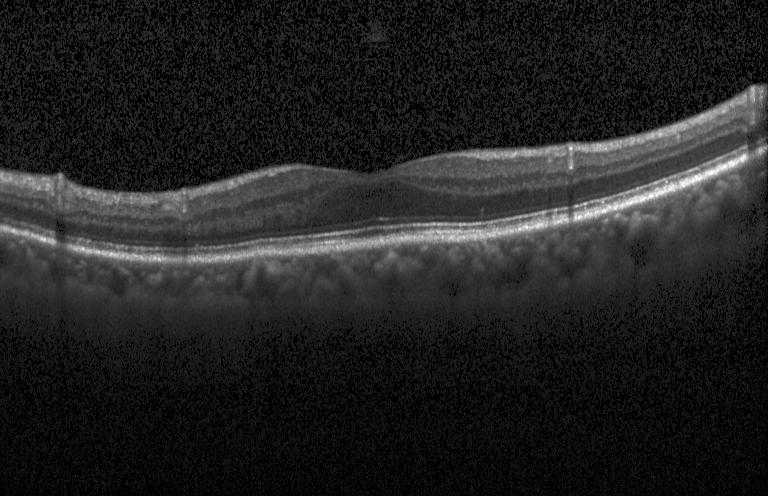

Macular OCT: no choroidal neovascularization, no diabetic macular edema, and no drusen.